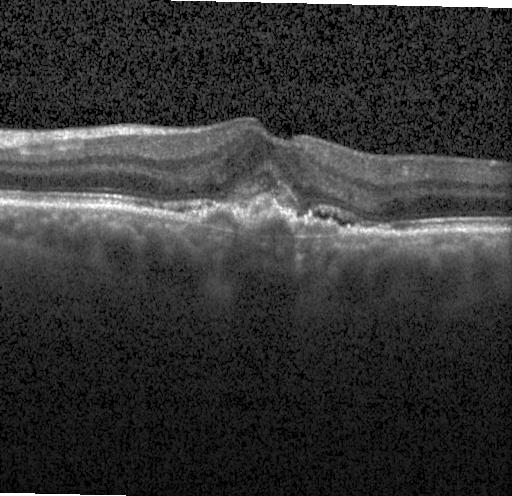

Spectral-domain OCT. Optical coherence tomography B-scan — Impression: CNV.